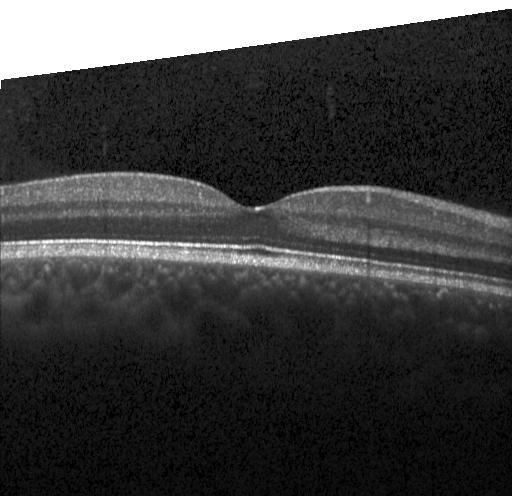 OCT B-scan; SD-OCT. Dx: neither choroidal neovascularization, diabetic macular edema, nor drusen.